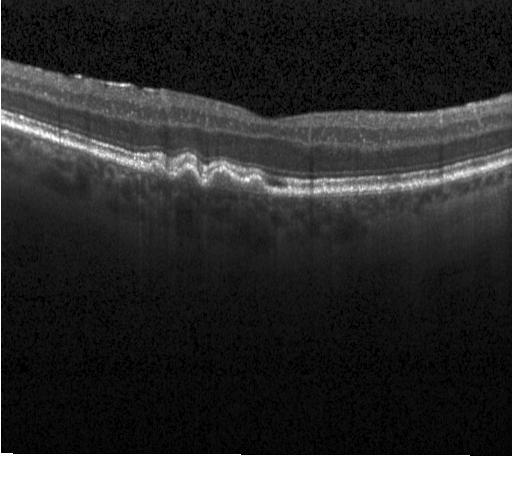

Acquired on a Heidelberg Spectralis; fovea-centered; optical coherence tomography B-scan
Diagnosis: multiple drusen.